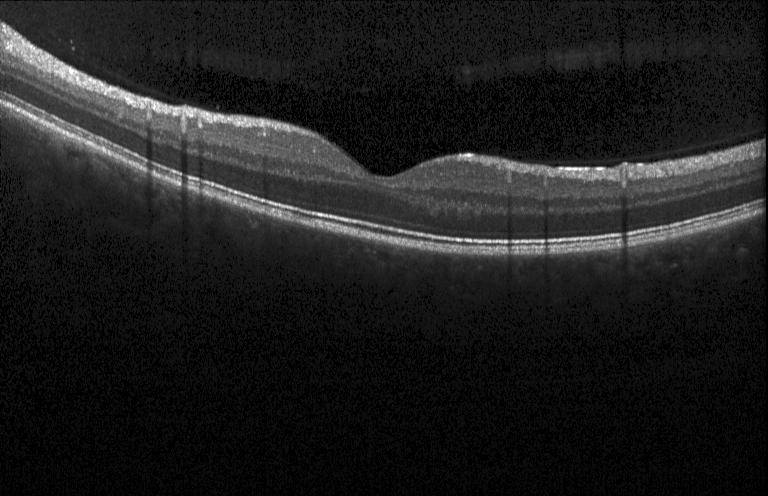

Spectral-domain OCT · Heidelberg Spectralis · optical coherence tomography B-scan · fovea-centered — Diagnosis: no evidence of CNV, DME, or drusen.